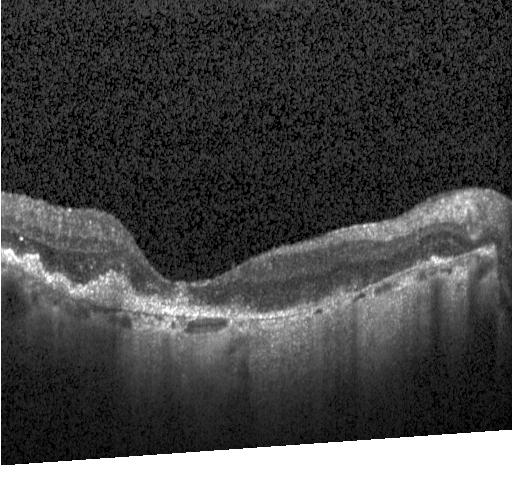 Retinal OCT cross-section
This B-scan demonstrates a choroidal neovascular membrane.